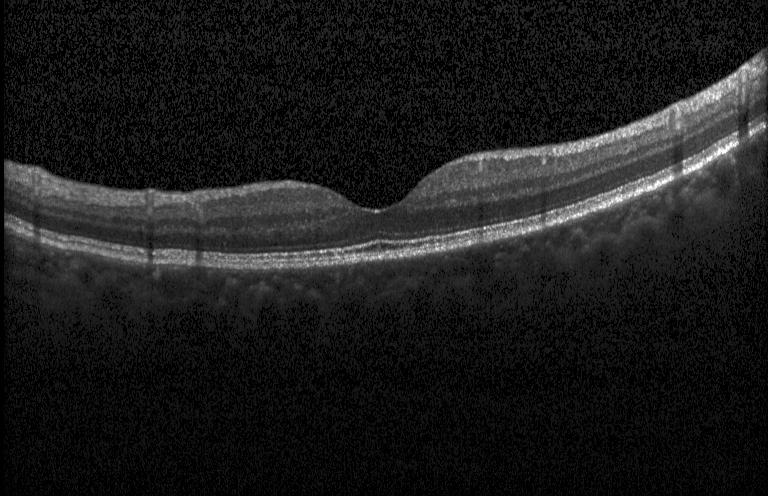

The scan shows neither choroidal neovascularization, diabetic macular edema, nor drusen.